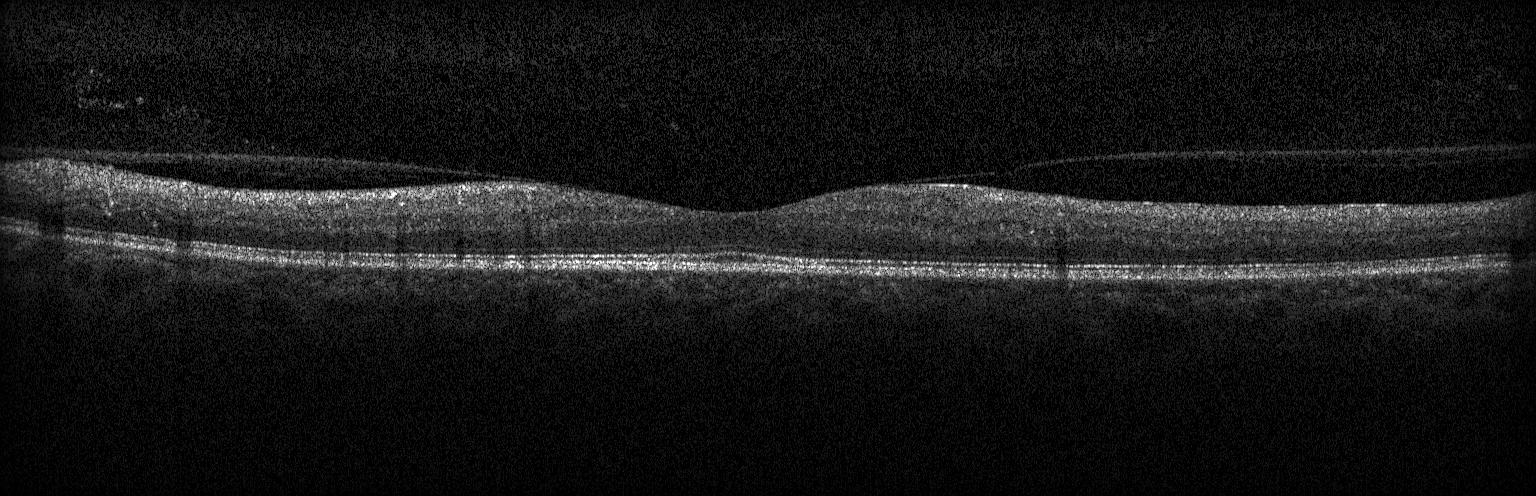 Assessment: no evidence of choroidal neovascularization, diabetic macular edema, or drusen.